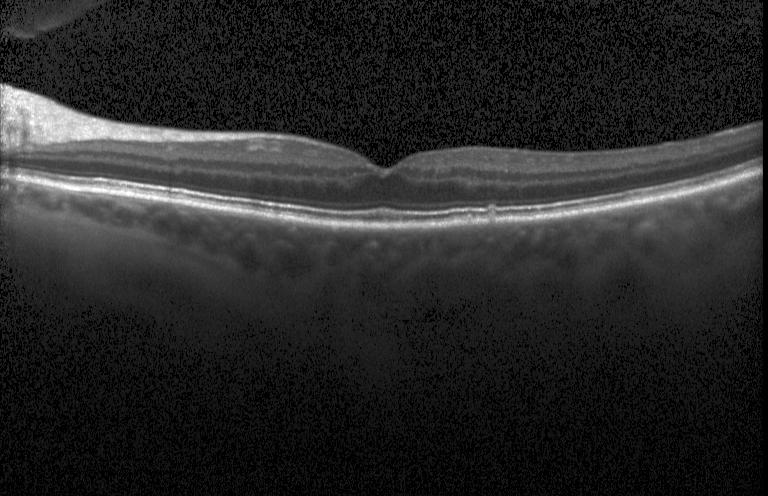
Macular OCT: multiple drusen.